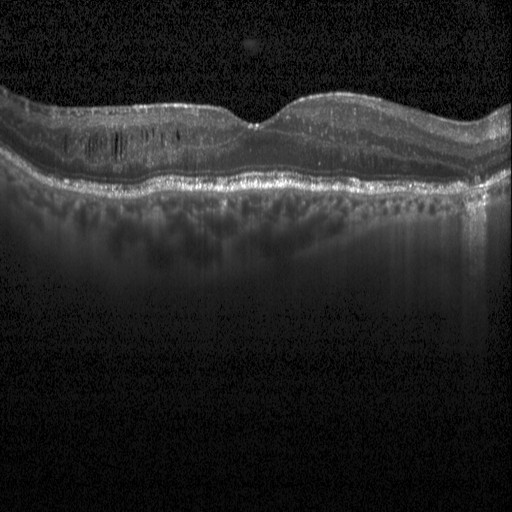

Optical coherence tomography B-scan
Diabetic macular edema (DME).